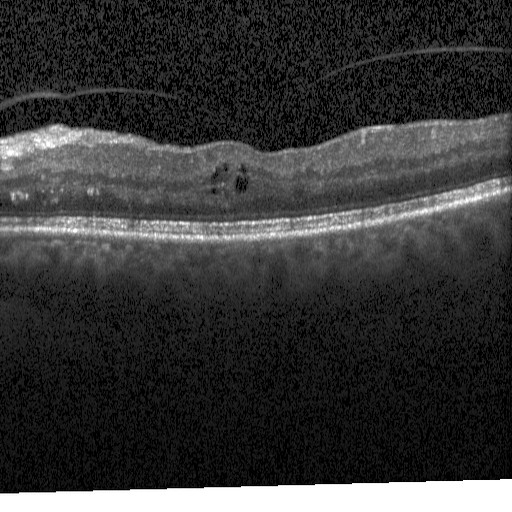

SD-OCT; instrument: Heidelberg Spectralis; OCT line scan.
Assessment: diabetic macular edema.